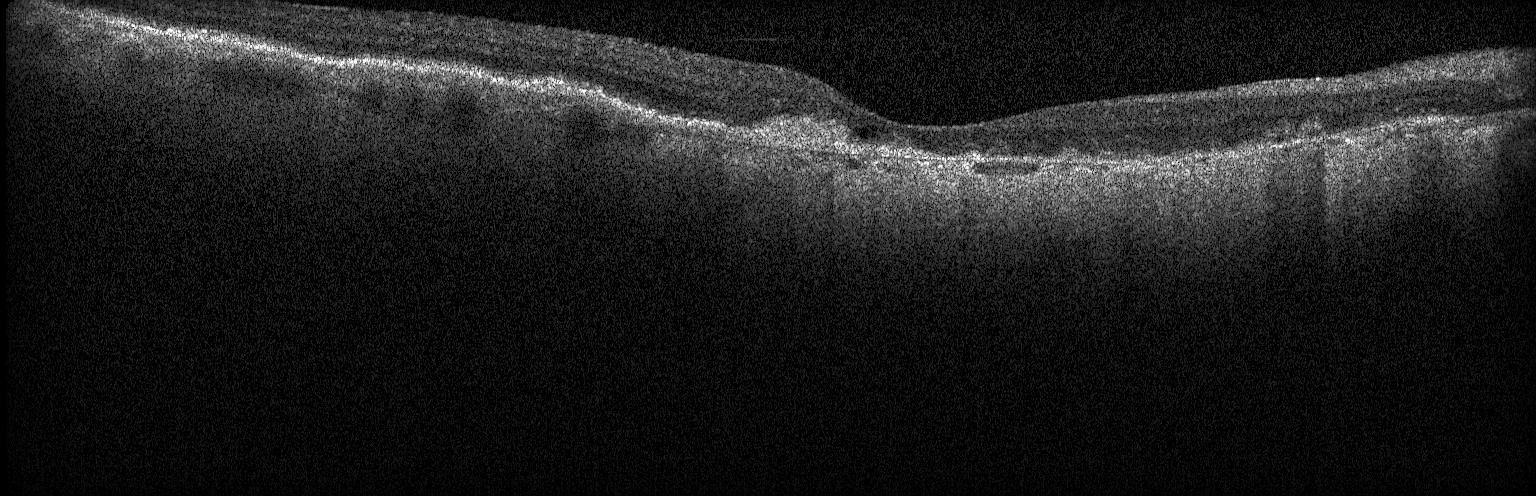

The scan shows a choroidal neovascular membrane.